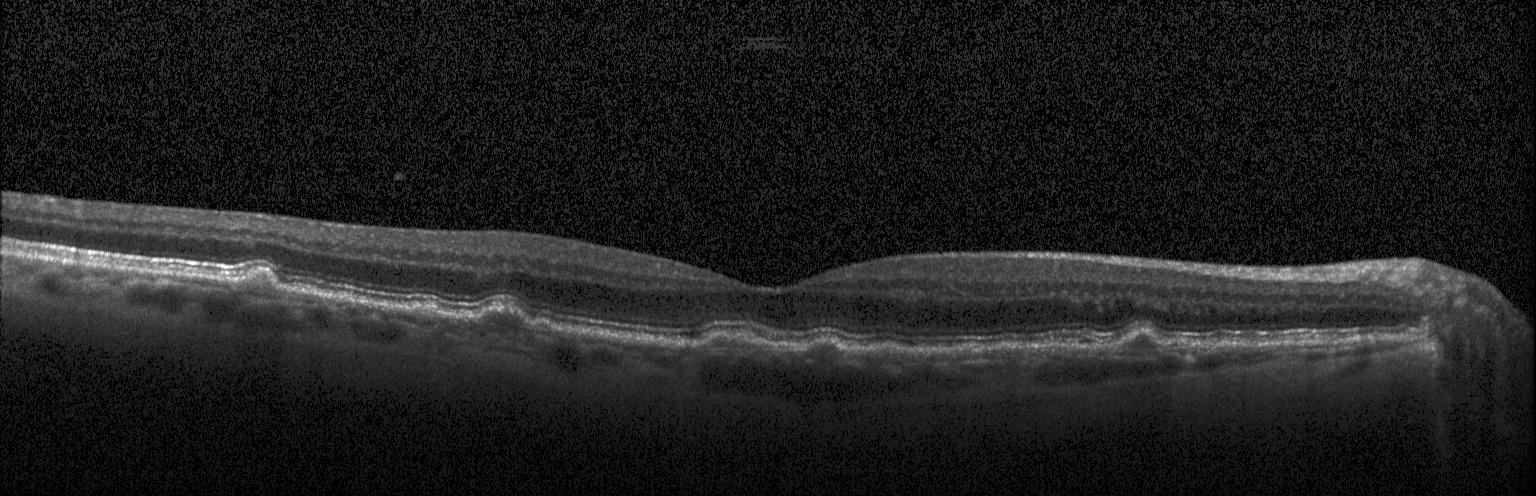

OCT finding: drusen.